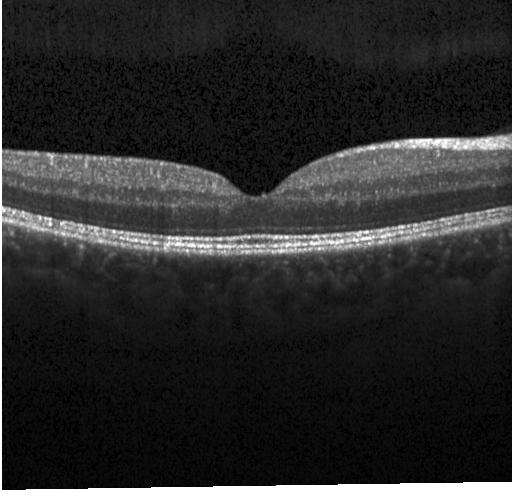 Through the macula; optical coherence tomography scan; Heidelberg Spectralis
Neither CNV, DME, nor drusen.